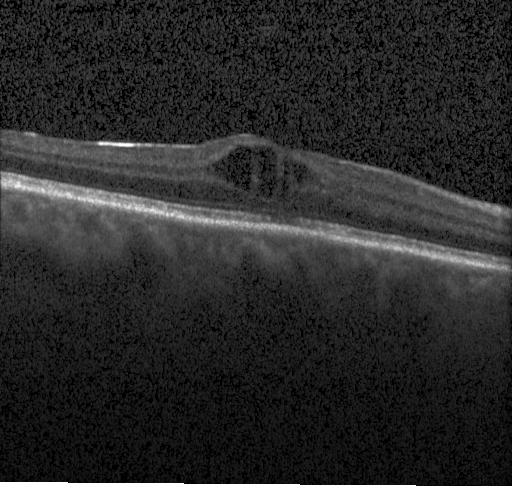
Finding: DME.